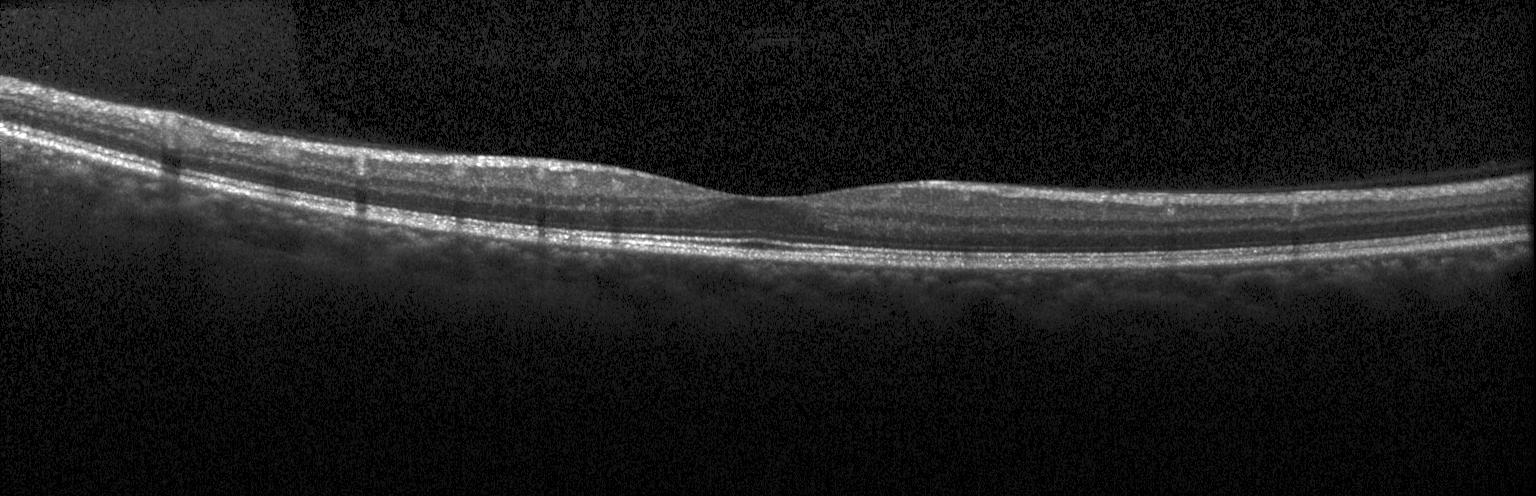
Heidelberg Spectralis, OCT B-scan. Impression: no choroidal neovascularization, diabetic macular edema, or drusen.